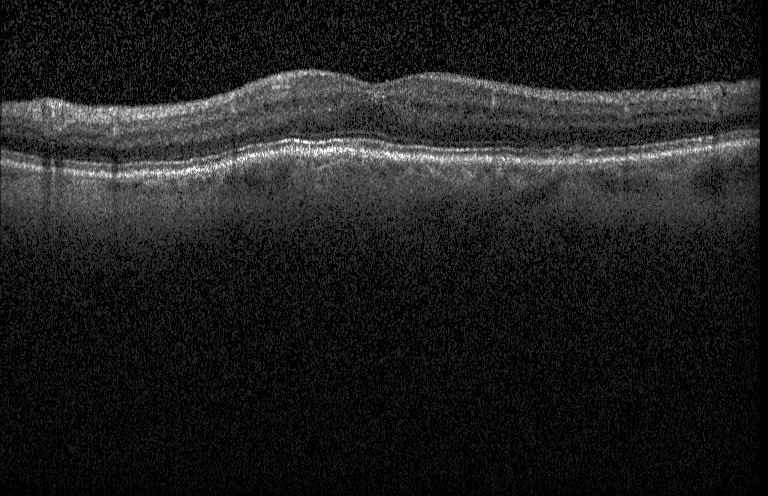
Diagnosis: no choroidal neovascularization, diabetic macular edema, or drusen.